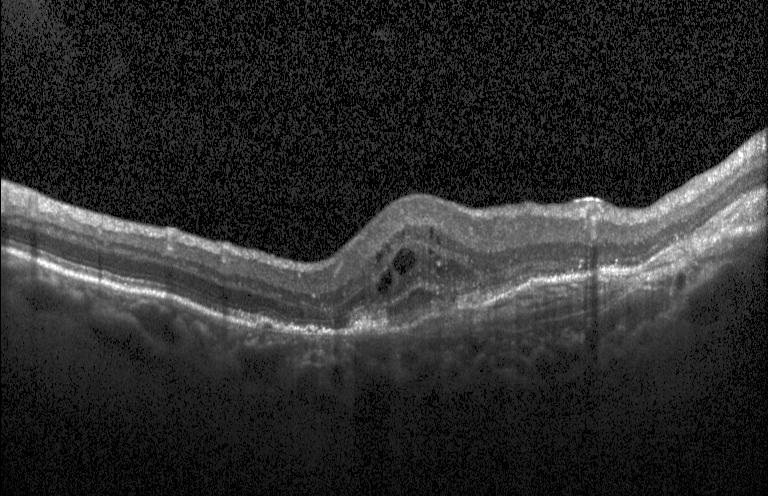 Dx: CNV.